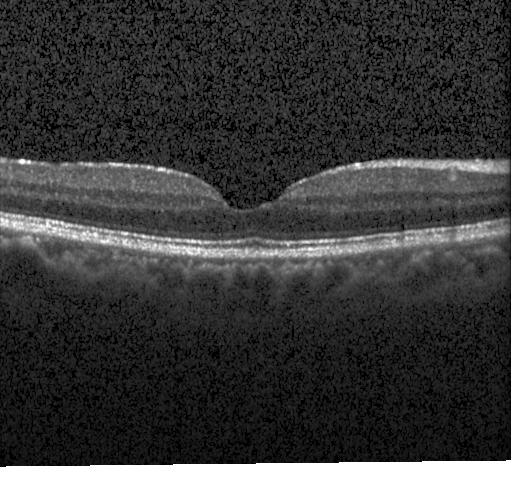

OCT line scan
Macular OCT: neither choroidal neovascularization, diabetic macular edema, nor drusen.